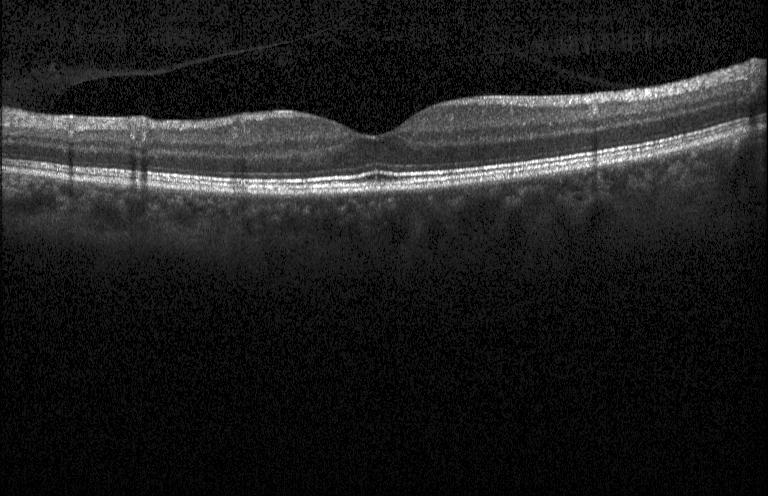 No choroidal neovascularization, no diabetic macular edema, and no drusen.